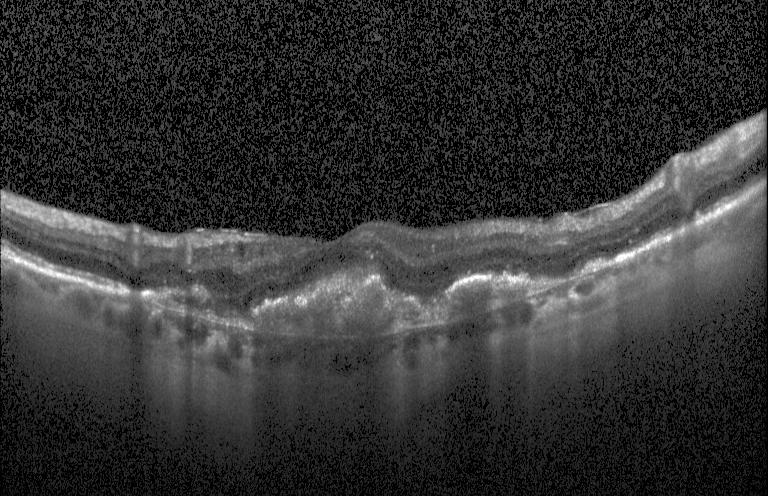 Impression: CNV.